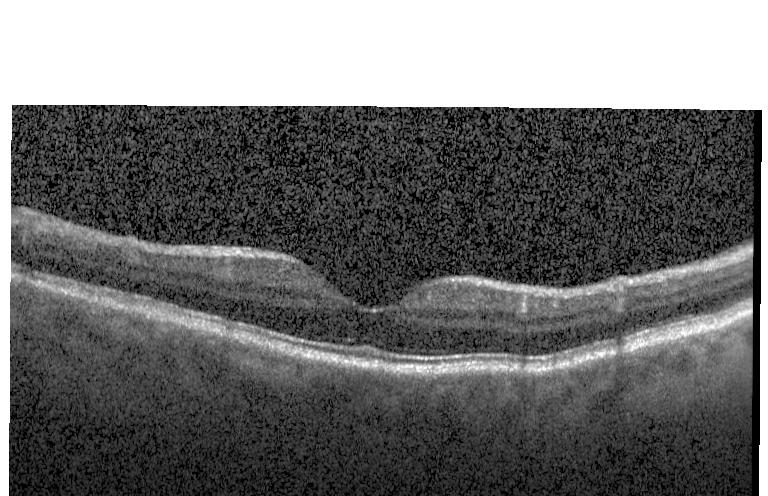

Diagnosis: no CNV, no DME, and no drusen.